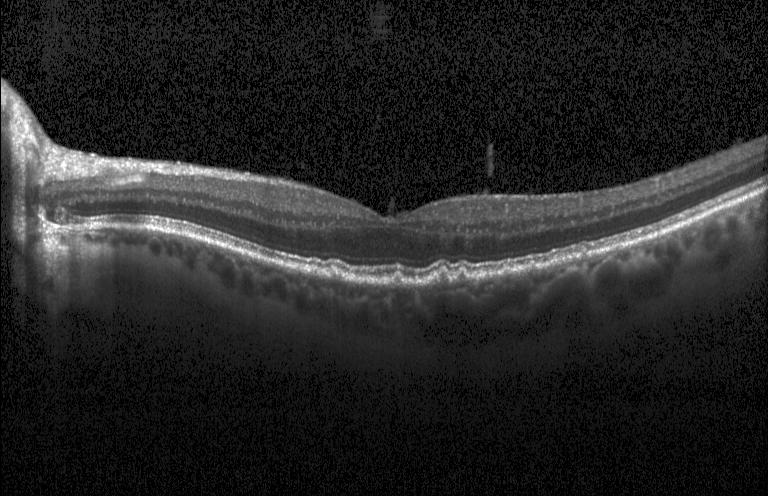

Drusen.